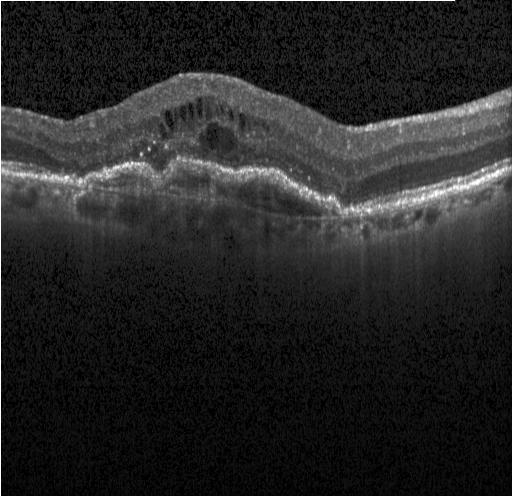 OCT scan showing choroidal neovascularization.